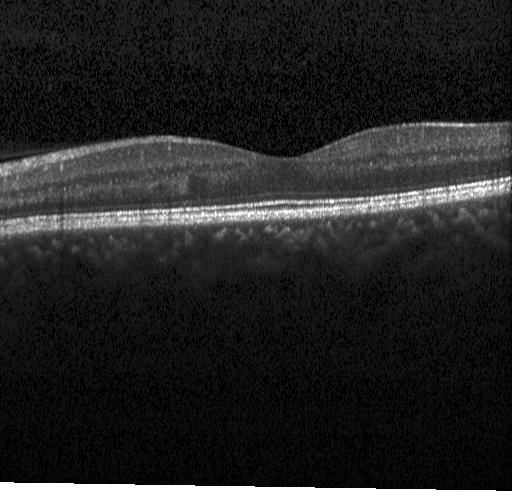
Retinal OCT B-scan
This B-scan demonstrates no evidence of CNV, DME, or drusen.